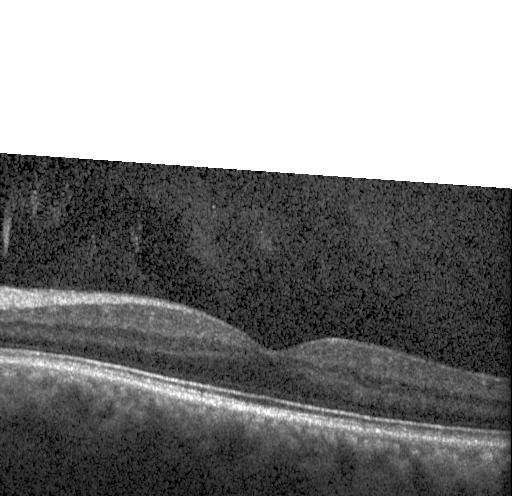 Macular OCT: neither choroidal neovascularization, diabetic macular edema, nor drusen.